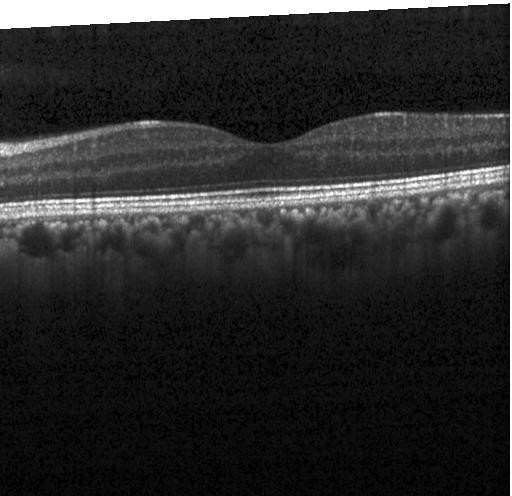
The scan shows neither choroidal neovascularization, diabetic macular edema, nor drusen.